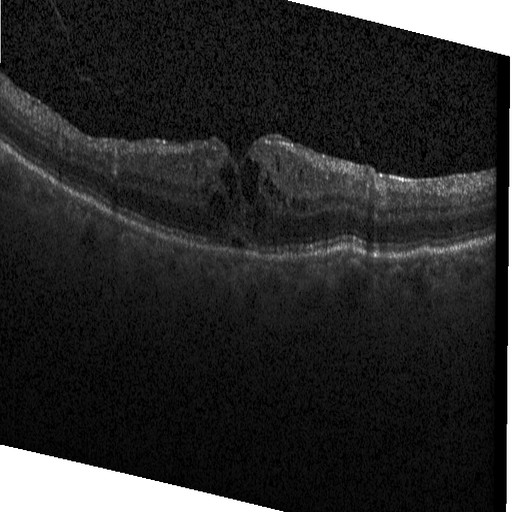

Macular OCT demonstrating diabetic macular edema.